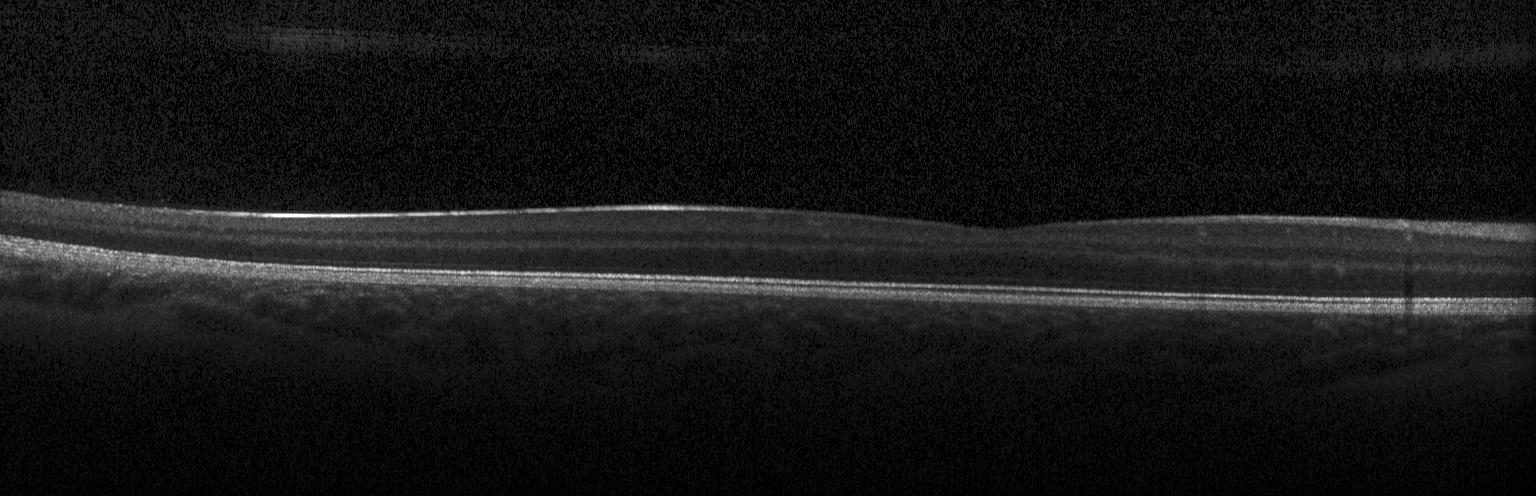
Optical coherence tomography scan
Impression: no evidence of choroidal neovascularization, diabetic macular edema, or drusen.